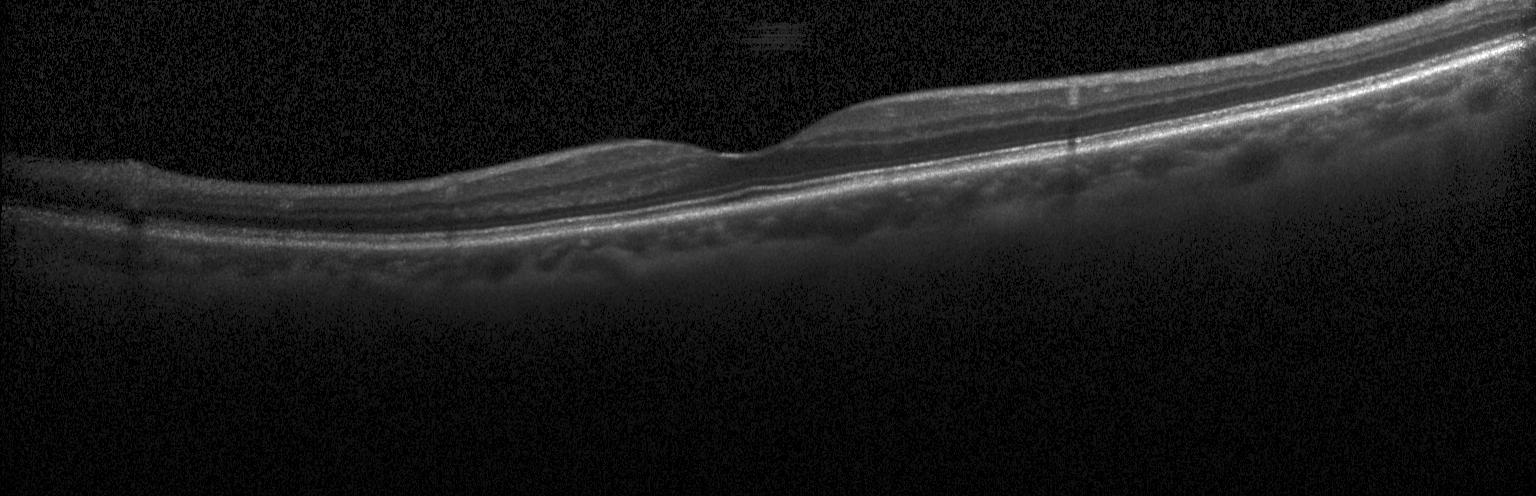
Optical coherence tomography scan · macular scan · instrument: Heidelberg Spectralis. This B-scan demonstrates neither CNV, DME, nor drusen.